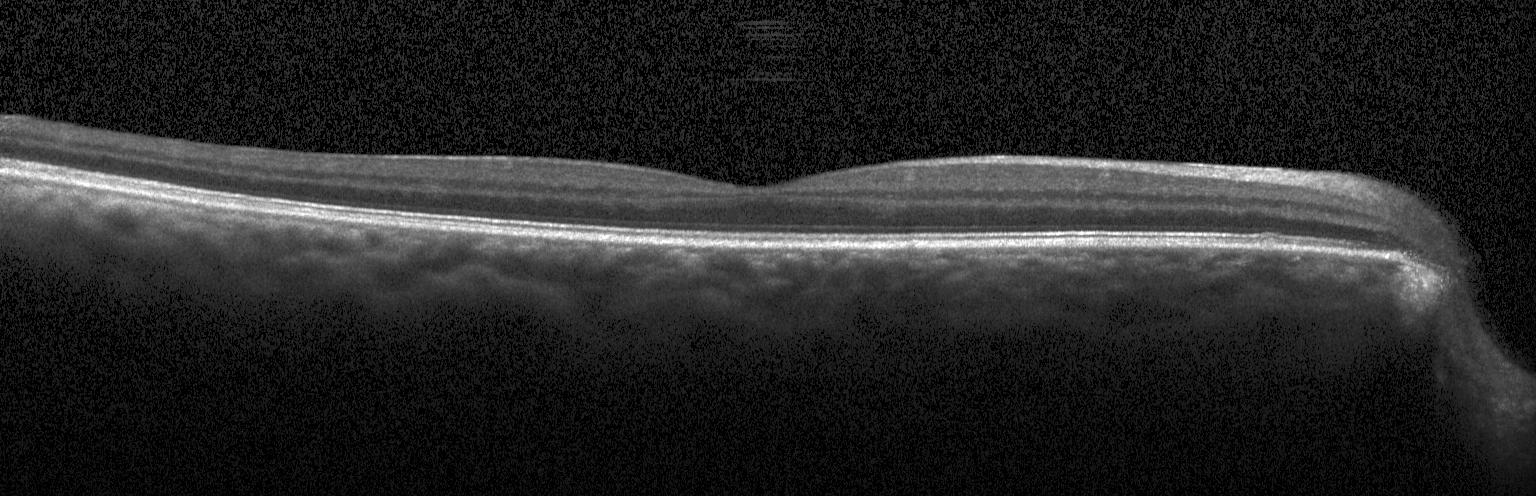 OCT scan showing no evidence of choroidal neovascularization, diabetic macular edema, or drusen.